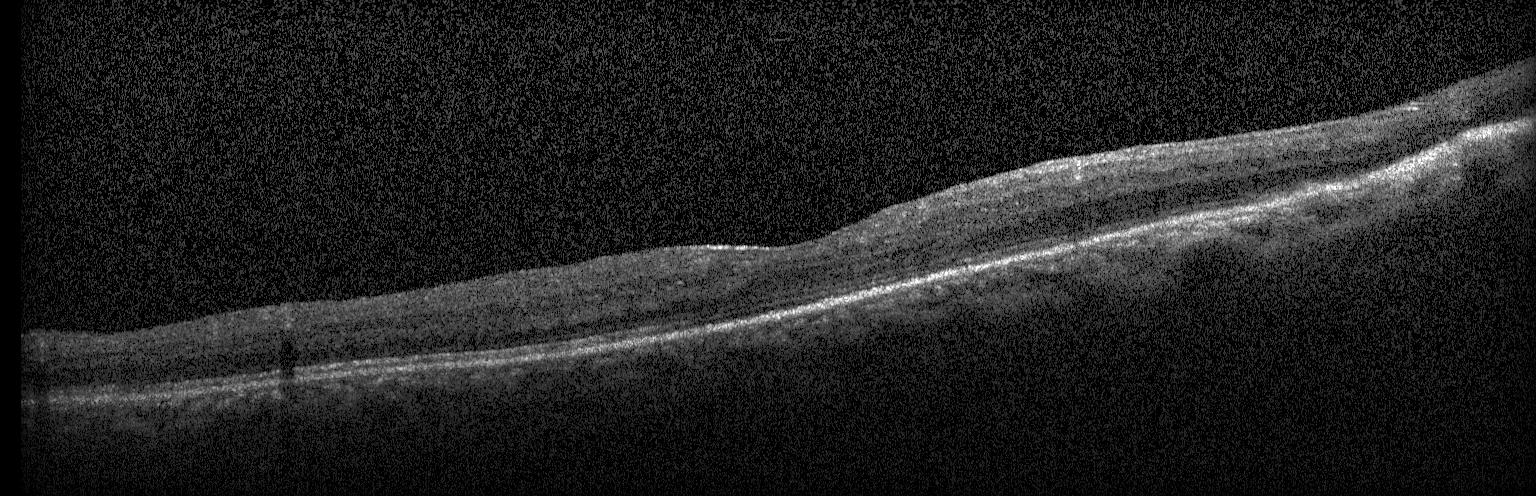
Diagnosis: no evidence of choroidal neovascularization, diabetic macular edema, or drusen.